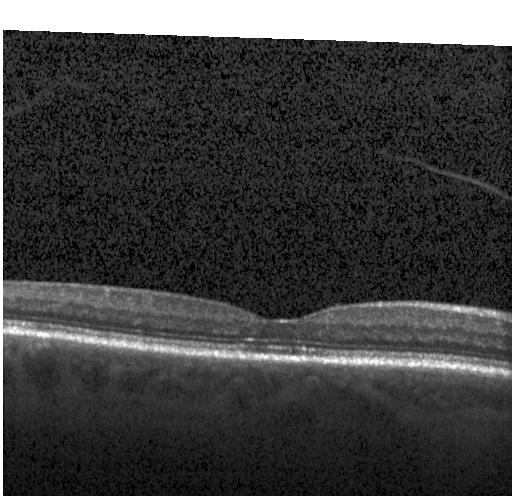

Optical coherence tomography B-scan · SD-OCT — Impression: no evidence of CNV, DME, or drusen.